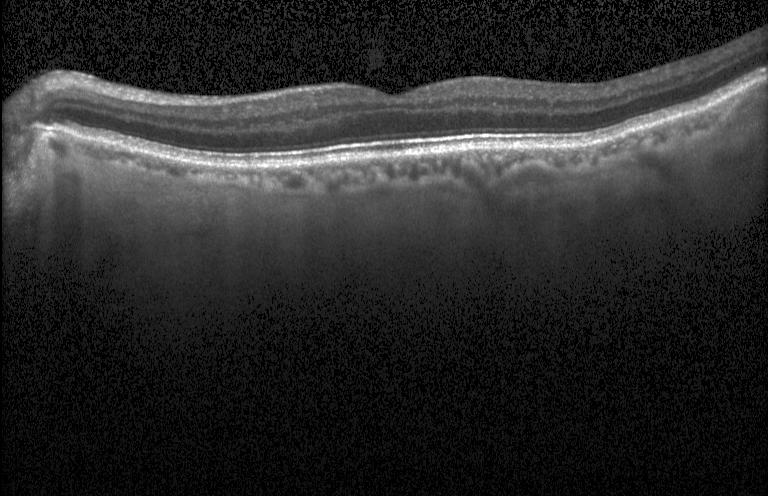

Impression: no choroidal neovascularization, diabetic macular edema, or drusen.